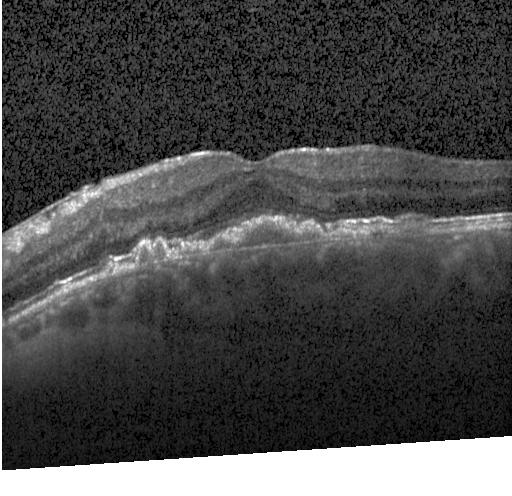 Macular OCT demonstrating choroidal neovascularization.